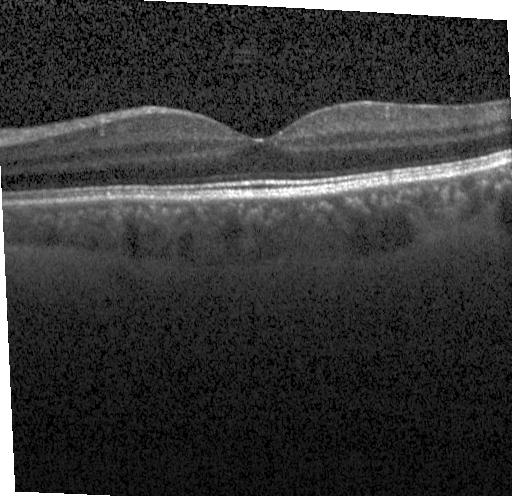
Macular OCT demonstrating no evidence of choroidal neovascularization, diabetic macular edema, or drusen.